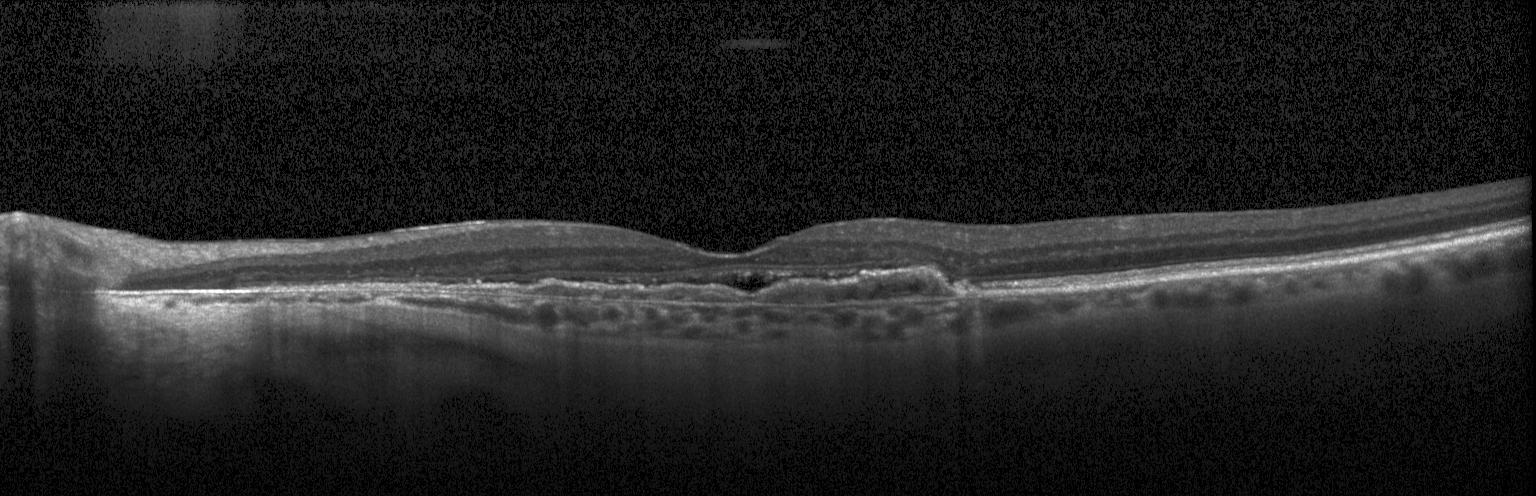 Heidelberg Spectralis, retinal OCT B-scan
Diagnosis: a choroidal neovascular membrane.